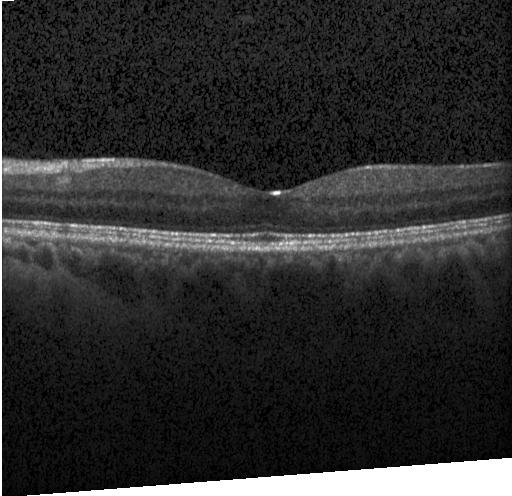
Optical coherence tomography B-scan.
Diagnosis: no evidence of CNV, DME, or drusen.